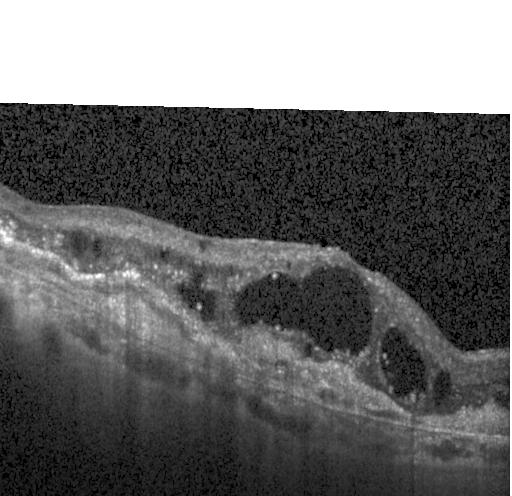
OCT B-scan showing a choroidal neovascular membrane.